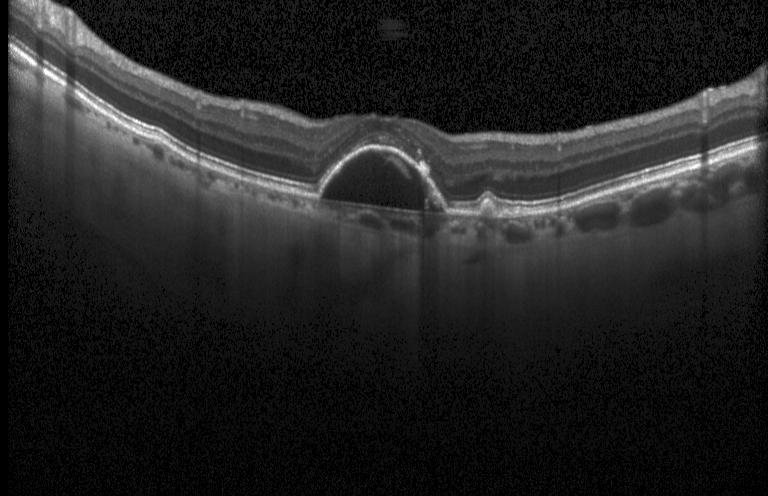 Spectral-domain OCT. OCT line scan — Finding: choroidal neovascularization.